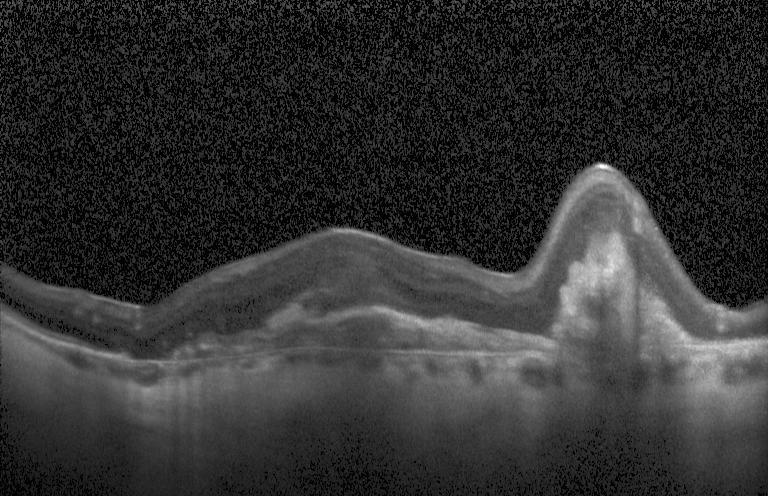 CNV.